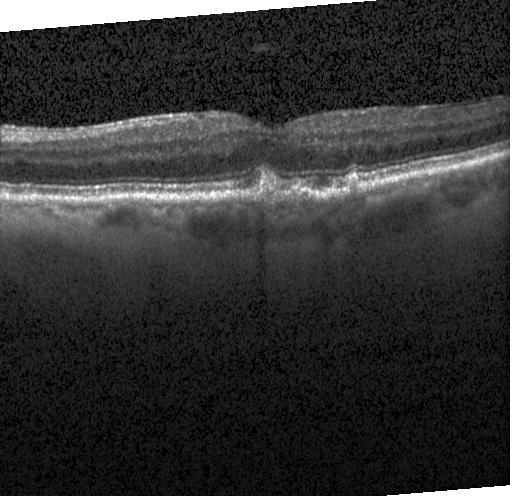
Diagnosis: drusen.